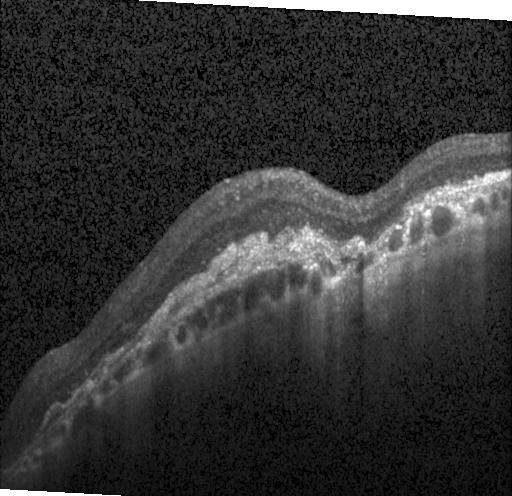

Fovea-centered. Heidelberg Spectralis OCT system. OCT B-scan — Dx: choroidal neovascularization.